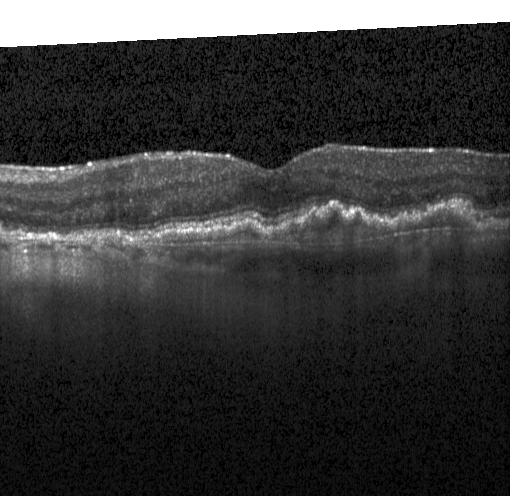
Optical coherence tomography B-scan
Impression: choroidal neovascularization.